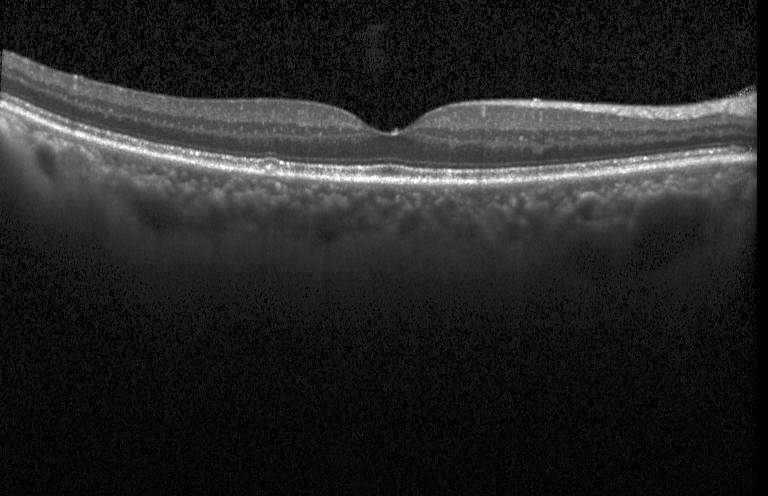

Macular OCT demonstrating multiple drusen.